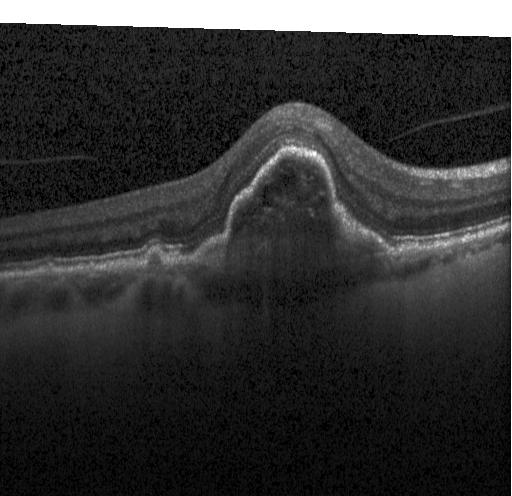
Impression: choroidal neovascularization.